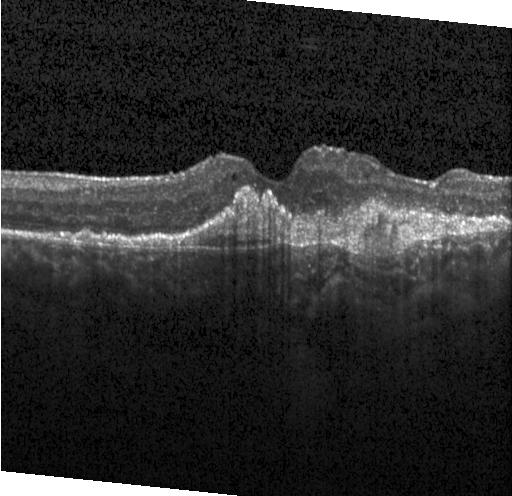
OCT line scan
Finding: a choroidal neovascular membrane.